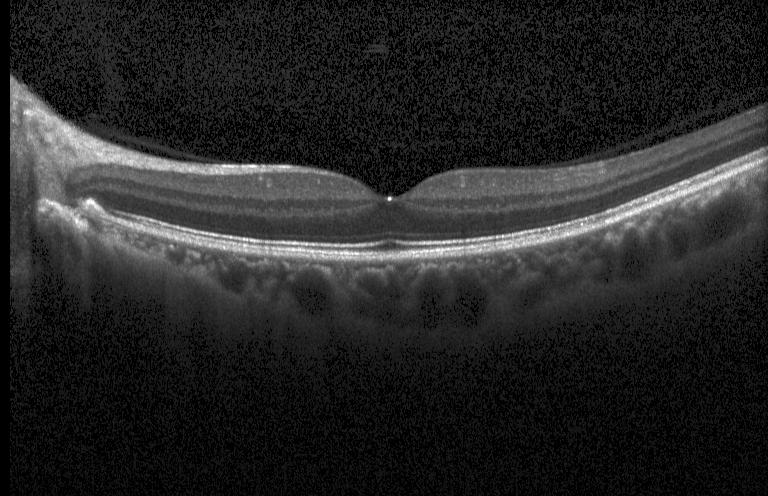
The scan shows no choroidal neovascularization, no diabetic macular edema, and no drusen.